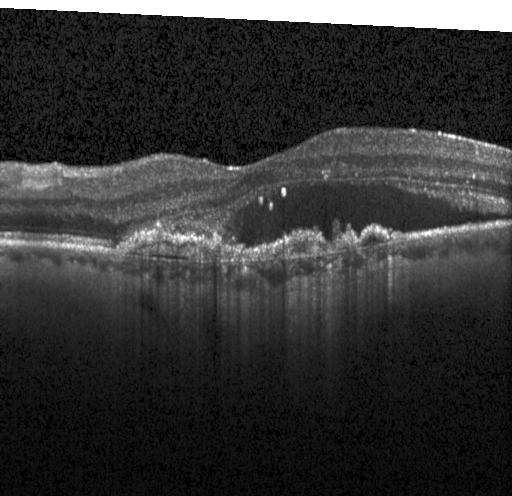
Assessment: a choroidal neovascular membrane.